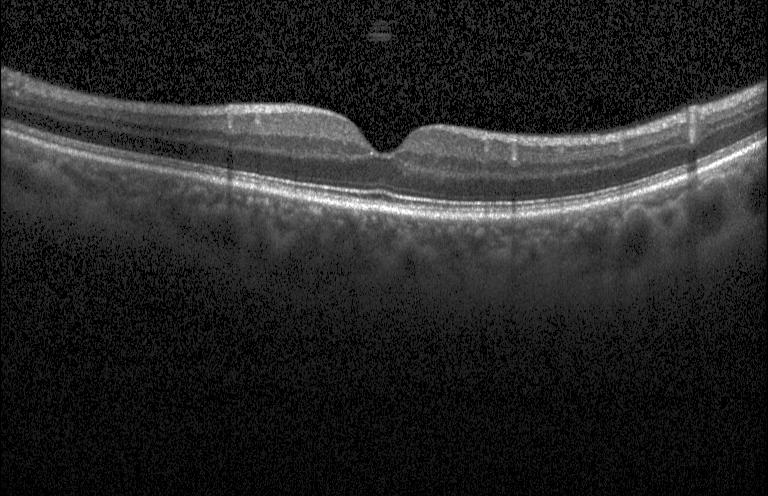

OCT B-scan.
Macular OCT: no evidence of choroidal neovascularization, diabetic macular edema, or drusen.